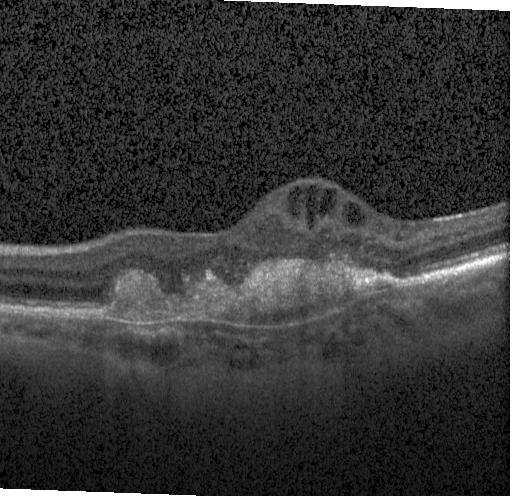 Centered on the fovea. Retinal OCT cross-section.
Impression: choroidal neovascularization.